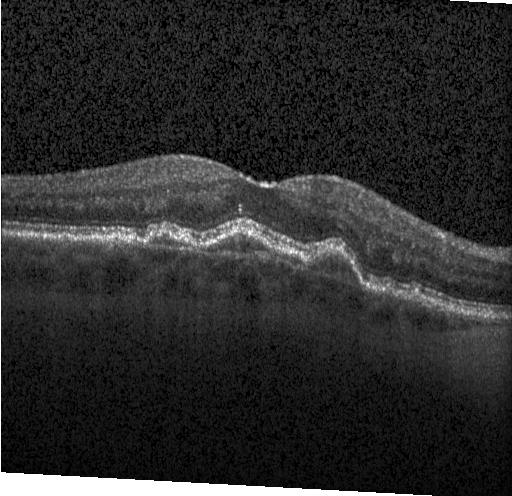
Heidelberg Spectralis · retinal OCT B-scan
Dx: CNV.